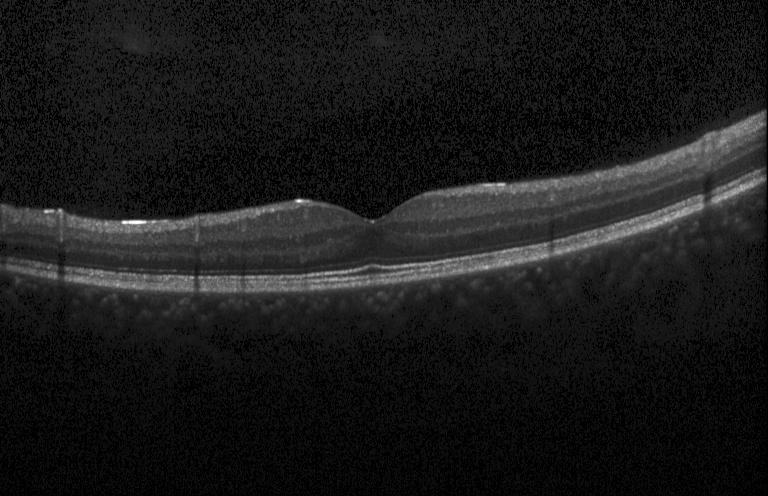
Optical coherence tomography B-scan. Centered on the fovea — Neither choroidal neovascularization, diabetic macular edema, nor drusen.